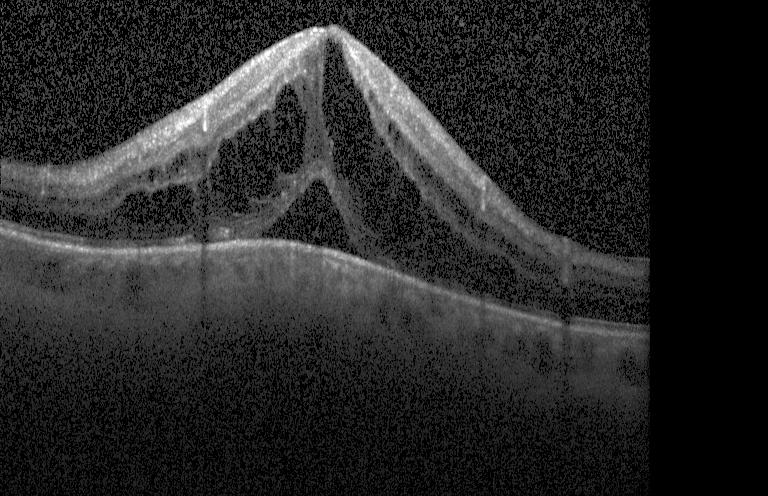
Retinal OCT B-scan · Heidelberg Spectralis OCT system
Diabetic macular edema (DME).